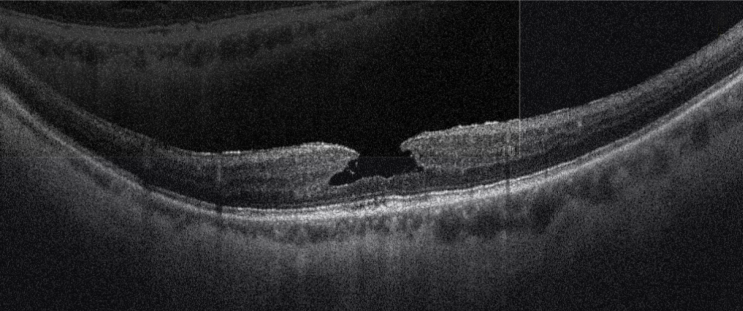 Impression: vitreomacular interface disease (VID).